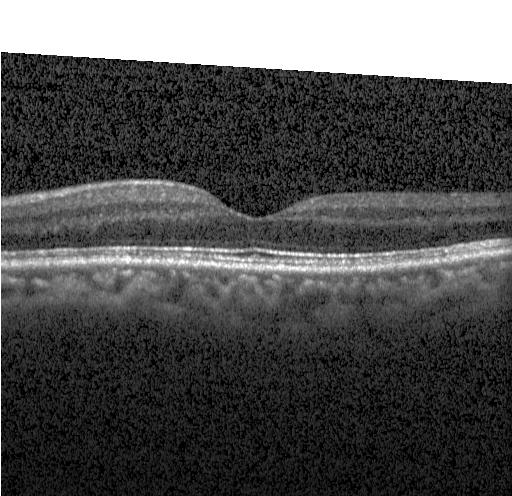 Finding: no evidence of choroidal neovascularization, diabetic macular edema, or drusen.